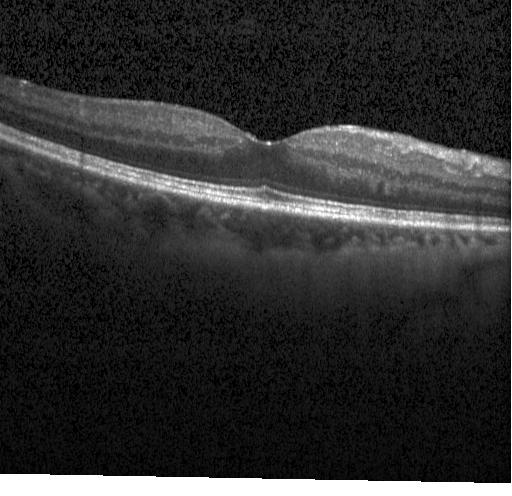

Through the macula; optical coherence tomography scan; SD-OCT.
OCT finding: no CNV, no DME, and no drusen.